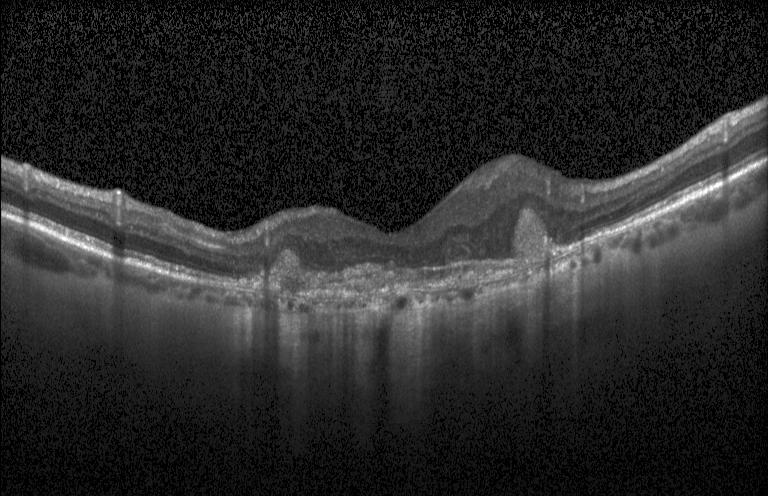 Dx: choroidal neovascularization.